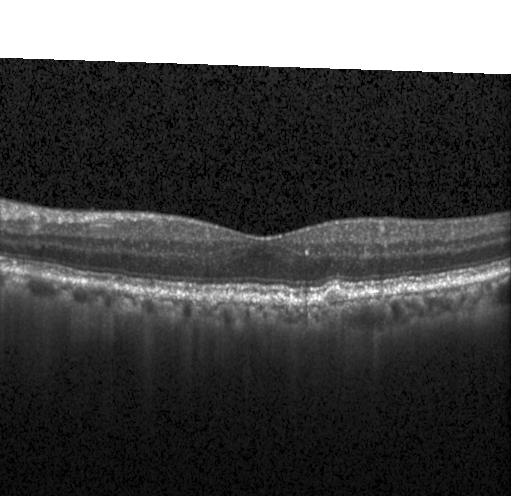 Heidelberg Spectralis; fovea-centered; OCT B-scan; spectral-domain OCT.
This B-scan demonstrates drusen.